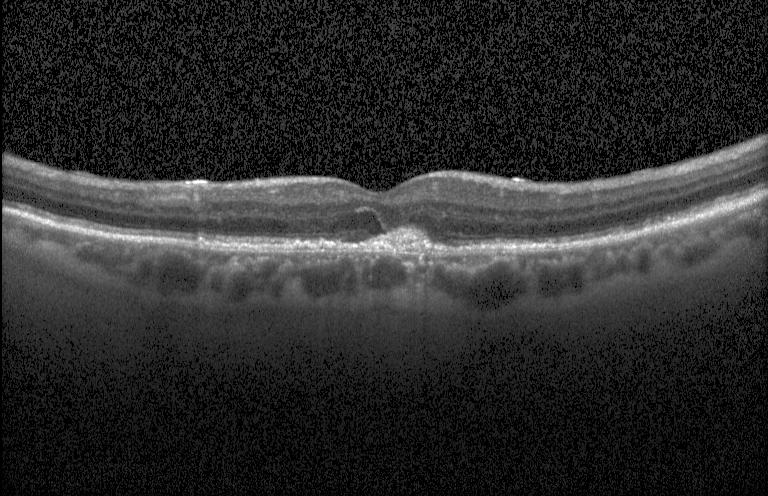 Fovea-centered · acquired on a Heidelberg Spectralis · OCT B-scan · spectral-domain OCT. A choroidal neovascular membrane.